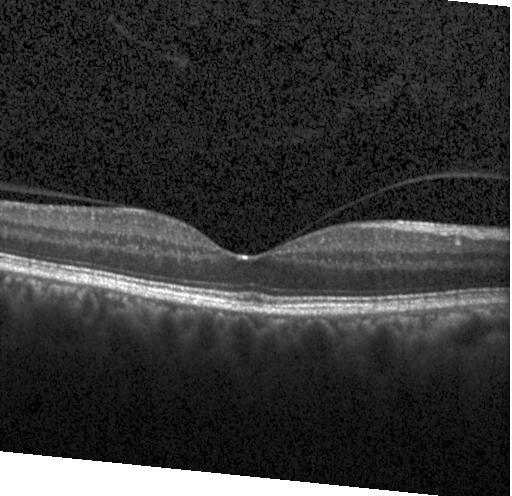
Diagnosis: no choroidal neovascularization, diabetic macular edema, or drusen.